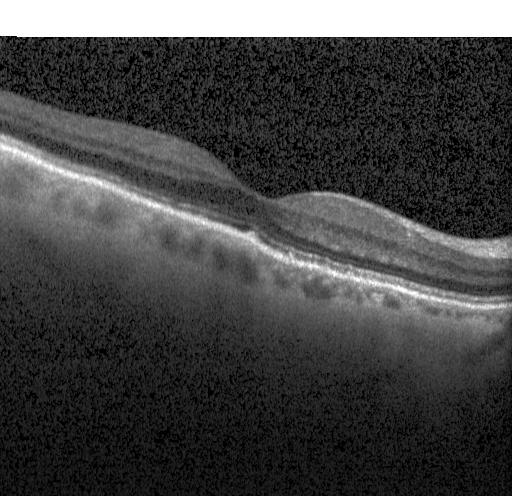

OCT line scan.
Impression: multiple drusen.